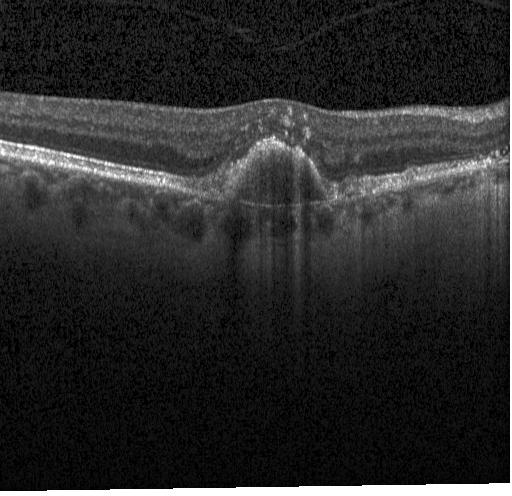 Impression: a choroidal neovascular membrane.